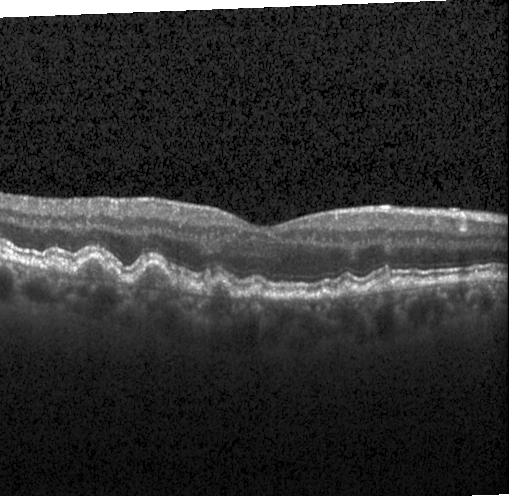 OCT line scan — This B-scan demonstrates drusen.